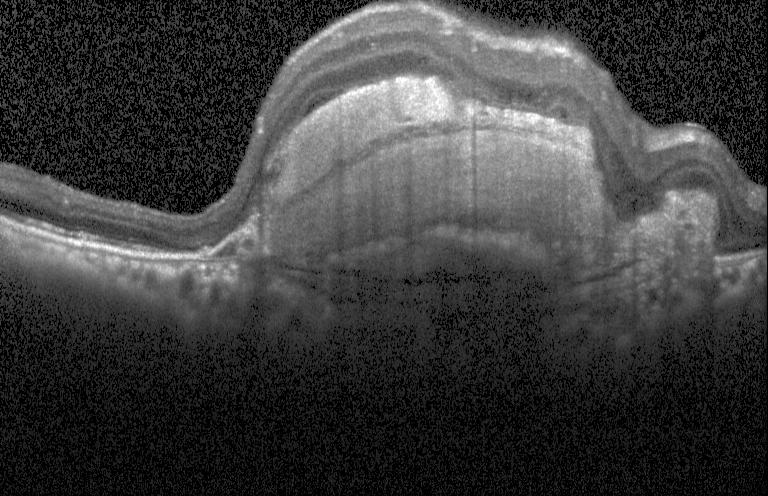

Retinal OCT B-scan
Impression: a choroidal neovascular membrane.